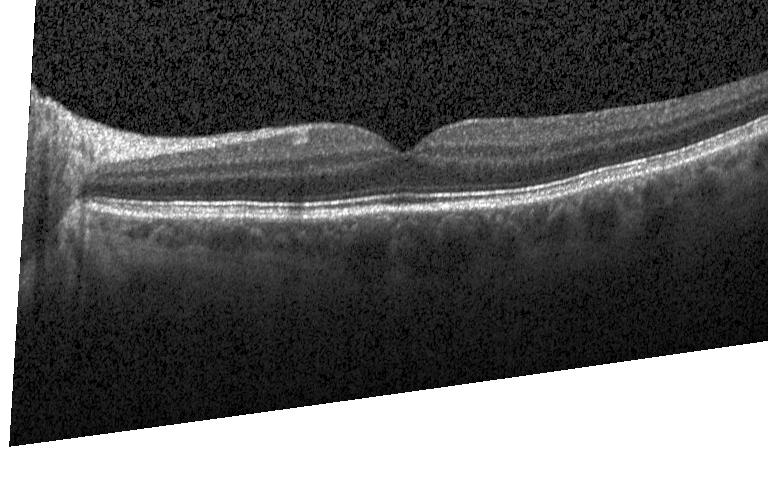

SD-OCT. Optical coherence tomography B-scan. Heidelberg Spectralis OCT system. Macular scan. This B-scan demonstrates no choroidal neovascularization, no diabetic macular edema, and no drusen.